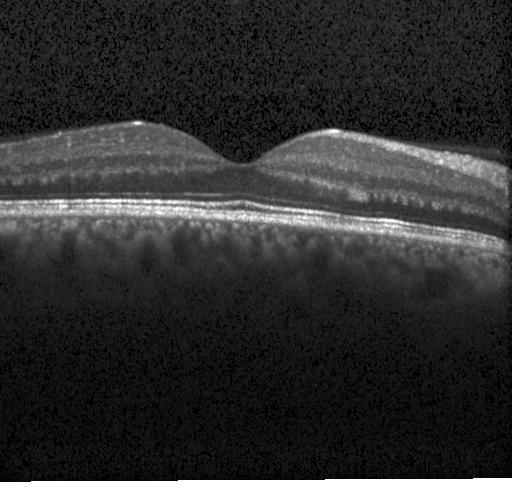

Heidelberg Spectralis OCT system, optical coherence tomography B-scan, through the macula, SD-OCT — Assessment: no CNV, DME, or drusen.